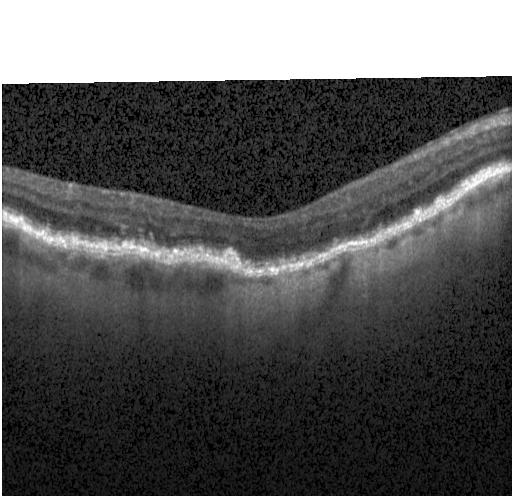 Retinal OCT cross-section, spectral-domain optical coherence tomography.
OCT finding: CNV.